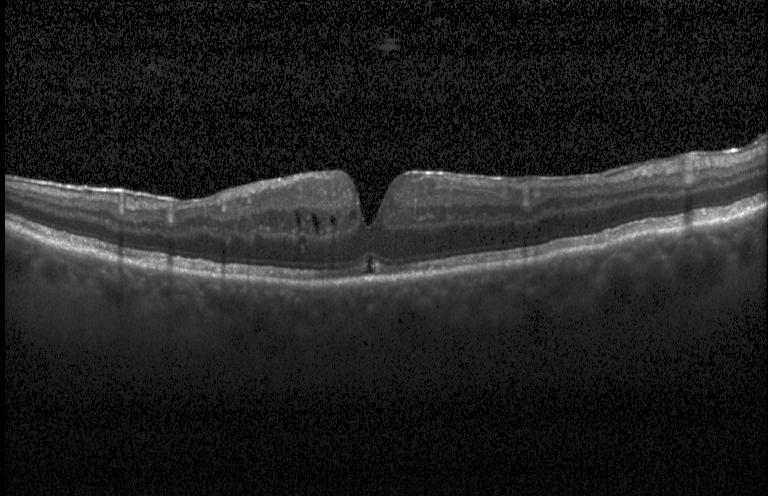

Optical coherence tomography scan.
This B-scan demonstrates DME.